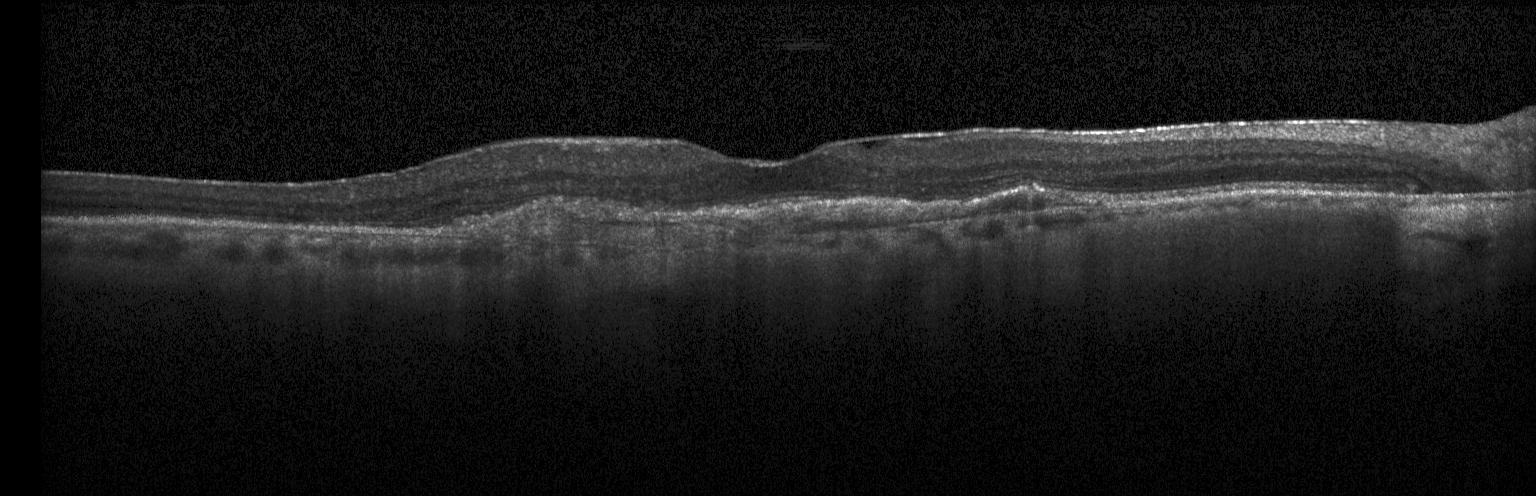

Finding: choroidal neovascularization.